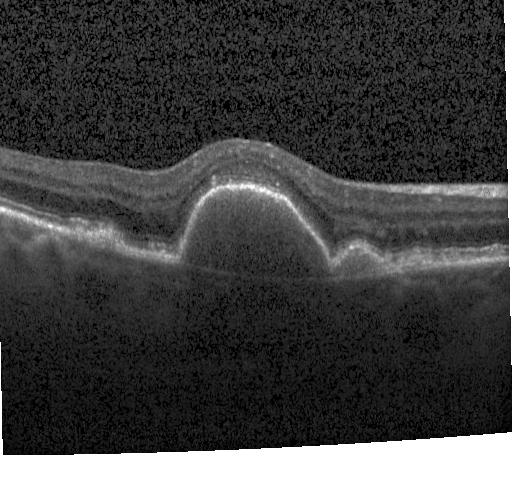
Retinal OCT B-scan; macular scan; Heidelberg Spectralis OCT system; spectral-domain OCT.
Assessment: choroidal neovascularization (CNV).